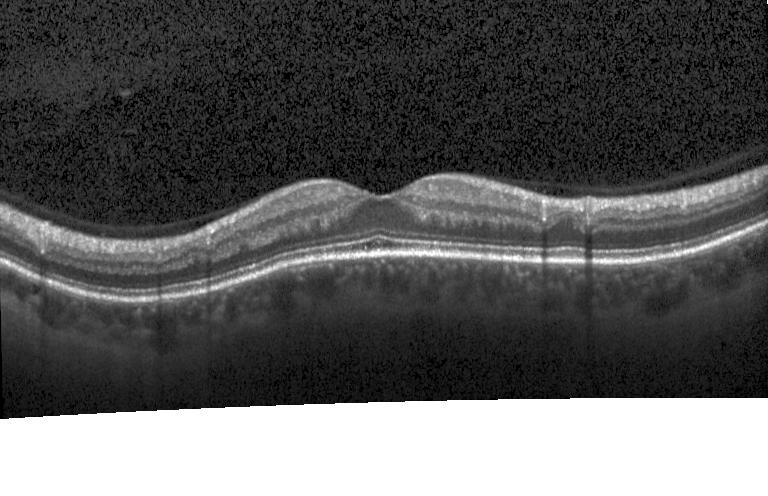 Impression: no choroidal neovascularization, no diabetic macular edema, and no drusen.